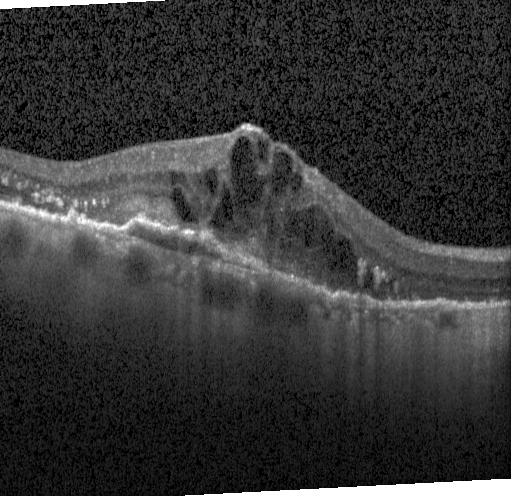 Retinal OCT B-scan. Centered on the fovea
Impression: a choroidal neovascular membrane.